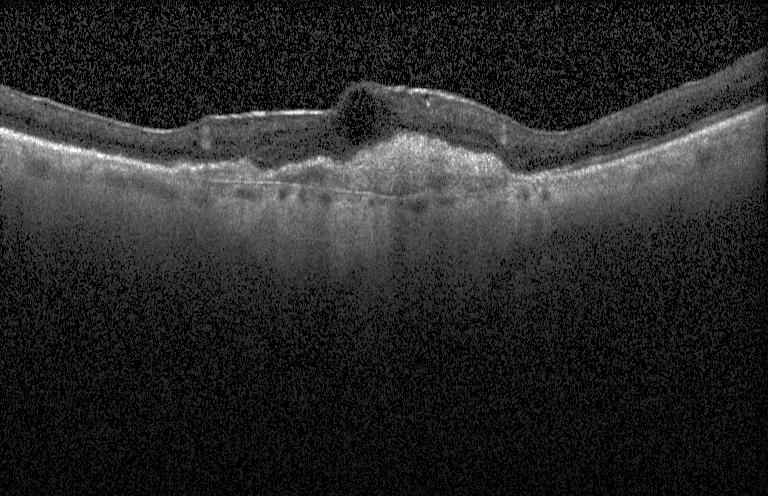

This B-scan demonstrates a choroidal neovascular membrane.